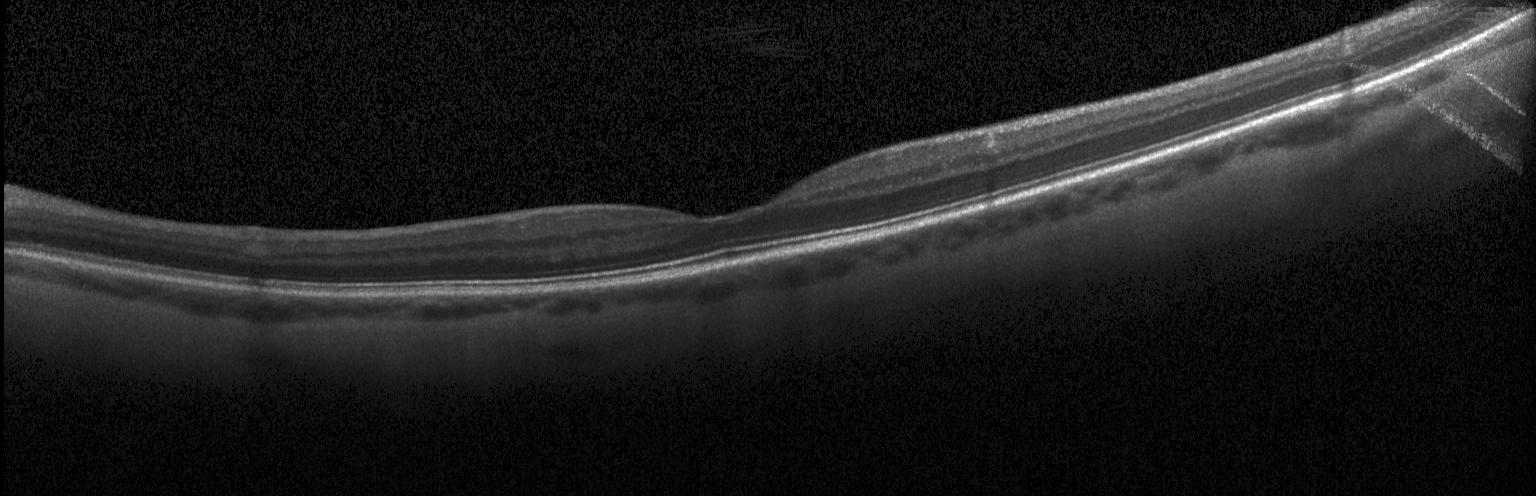
This B-scan demonstrates neither CNV, DME, nor drusen.